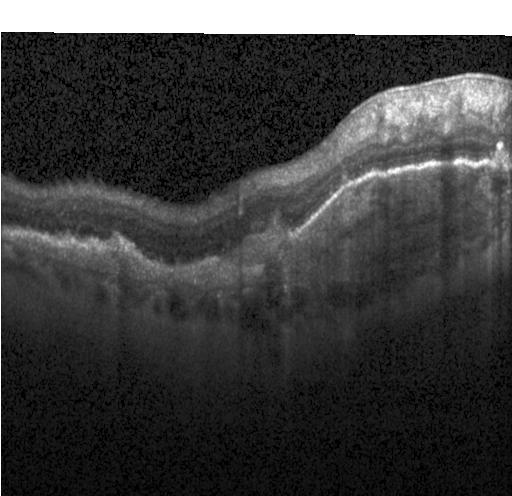 Macular OCT: a choroidal neovascular membrane.